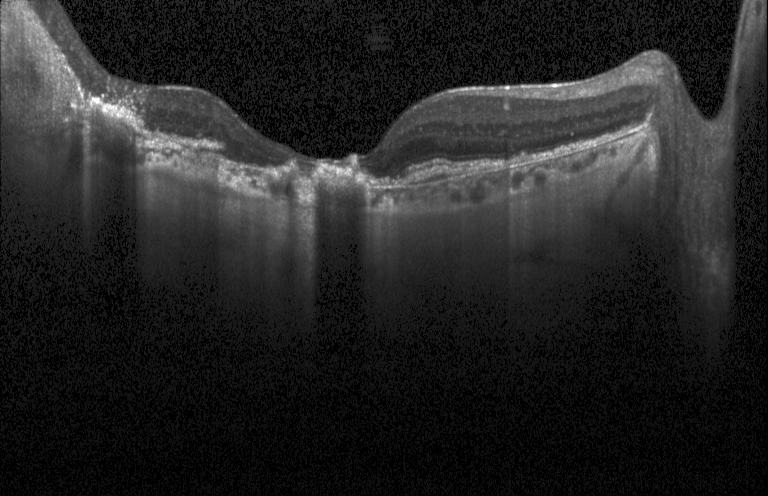

Instrument: Heidelberg Spectralis; SD-OCT; retinal OCT B-scan.
Assessment: choroidal neovascularization (CNV).